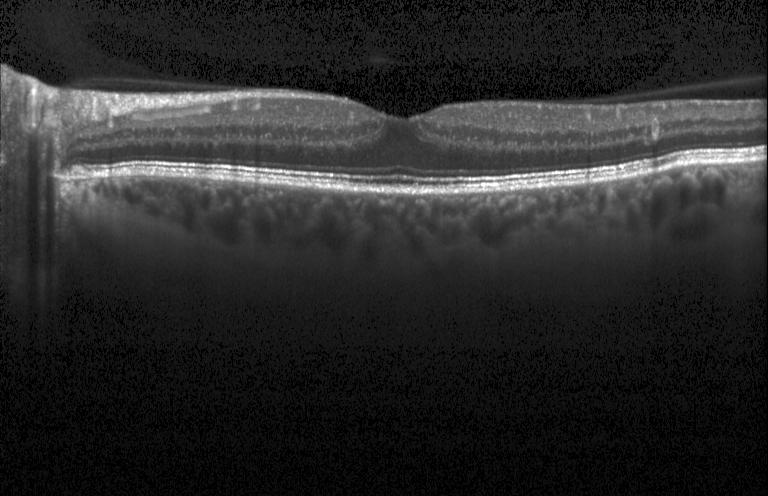 OCT line scan · spectral-domain optical coherence tomography · macular scan · acquired on a Heidelberg Spectralis. No choroidal neovascularization, diabetic macular edema, or drusen.